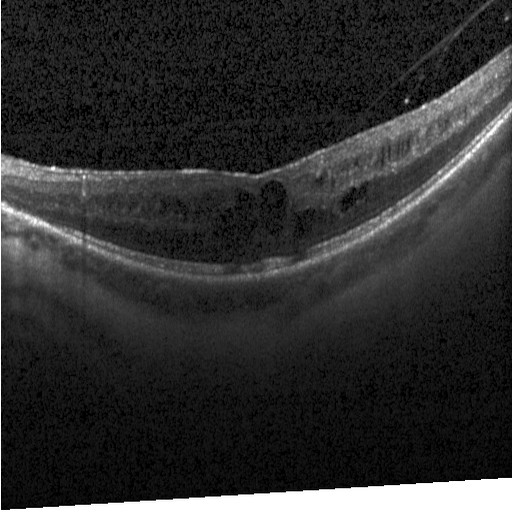
Spectral-domain OCT B-scan: diabetic macular edema (DME).